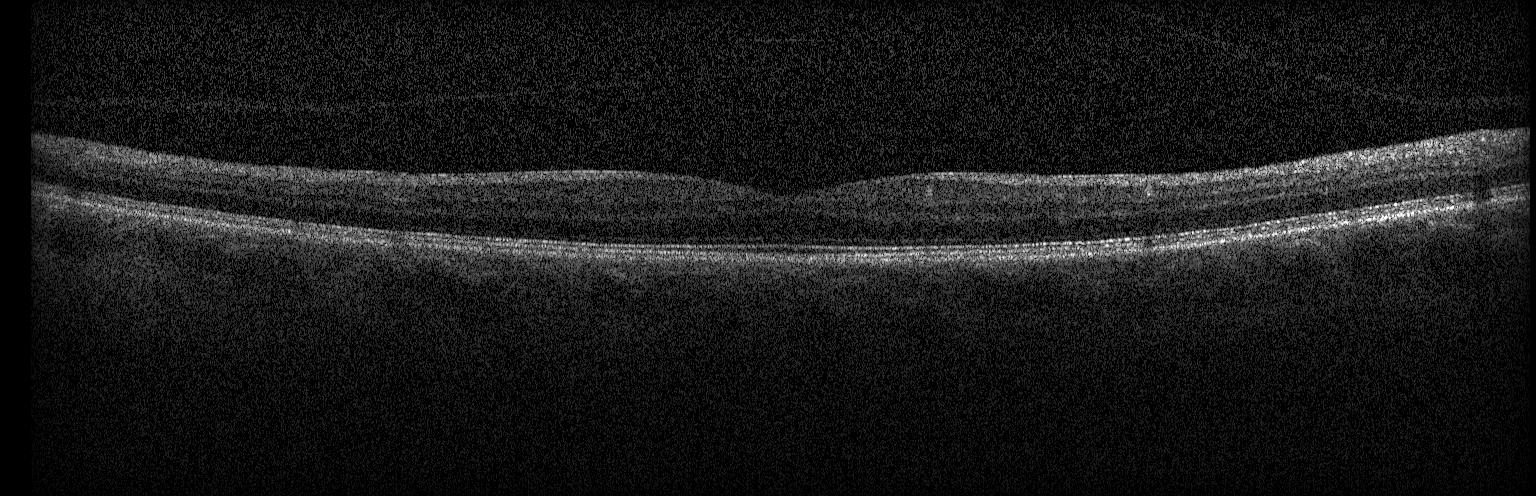

OCT line scan, acquired on a Heidelberg Spectralis, through the macula, spectral-domain optical coherence tomography
Finding: no choroidal neovascularization, no diabetic macular edema, and no drusen.